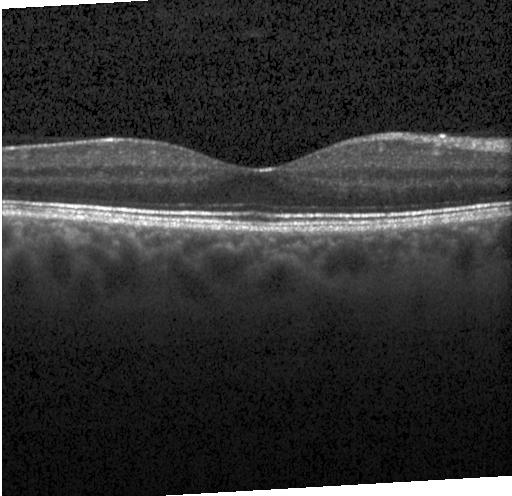

Instrument: Heidelberg Spectralis · retinal OCT cross-section — Dx: no CNV, DME, or drusen.